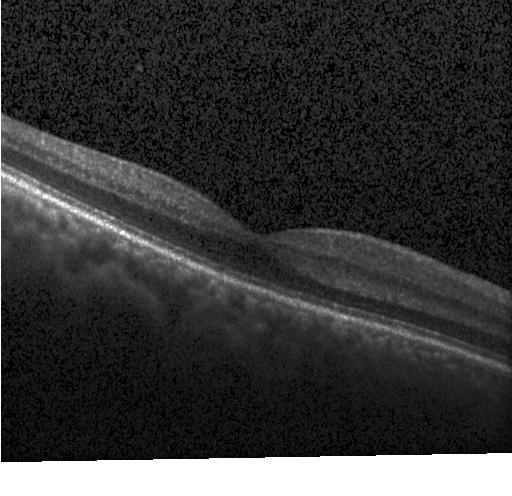

Centered on the fovea, optical coherence tomography B-scan, acquired on a Heidelberg Spectralis, spectral-domain OCT.
OCT finding: neither CNV, DME, nor drusen.